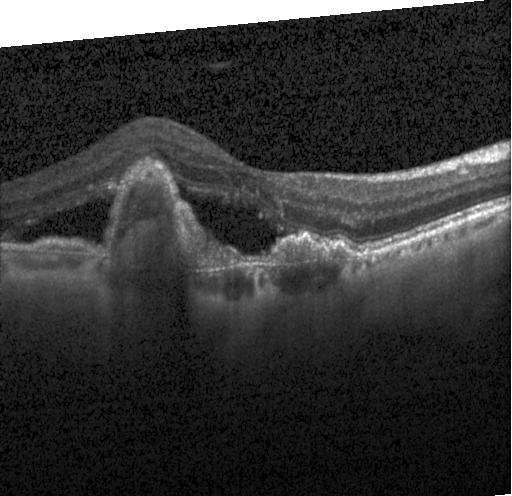
This B-scan demonstrates a choroidal neovascular membrane.